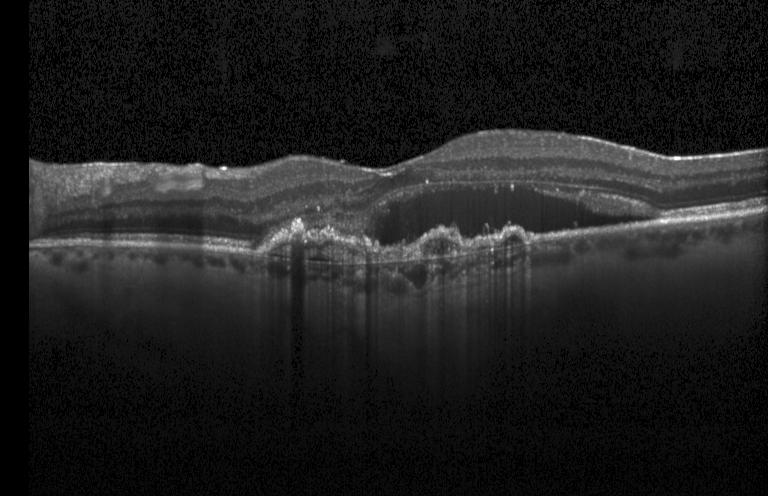

This B-scan demonstrates a choroidal neovascular membrane.